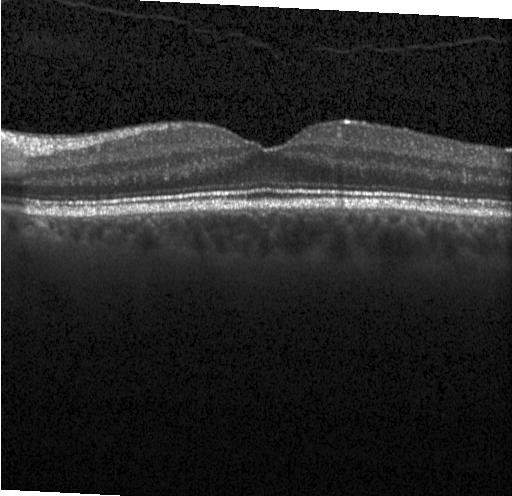
Heidelberg Spectralis OCT system; optical coherence tomography B-scan; through the macula; spectral-domain OCT
Impression: neither CNV, DME, nor drusen.